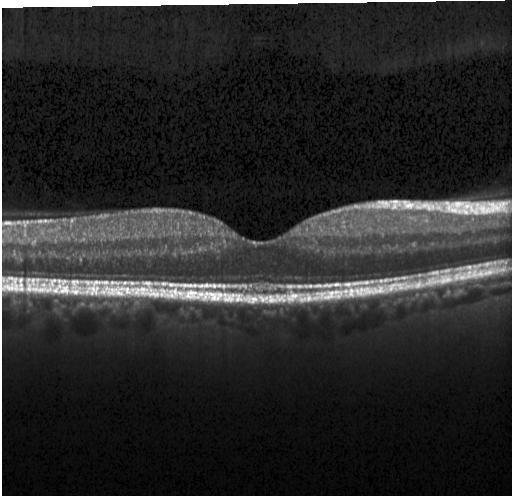 Optical coherence tomography B-scan. Spectral-domain optical coherence tomography. Instrument: Heidelberg Spectralis. Horizontal scan through the fovea
Diagnosis: no choroidal neovascularization, no diabetic macular edema, and no drusen.